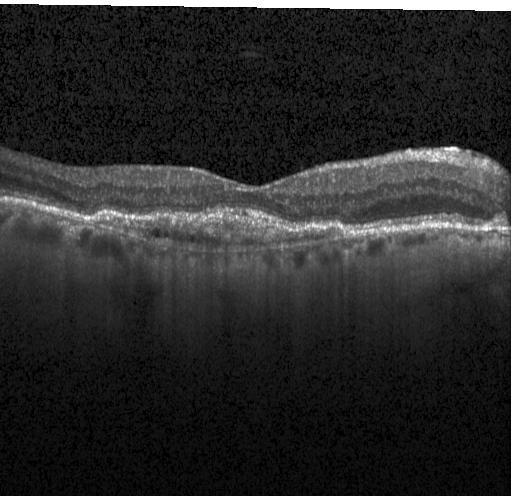

Retinal OCT B-scan. Assessment: choroidal neovascularization.